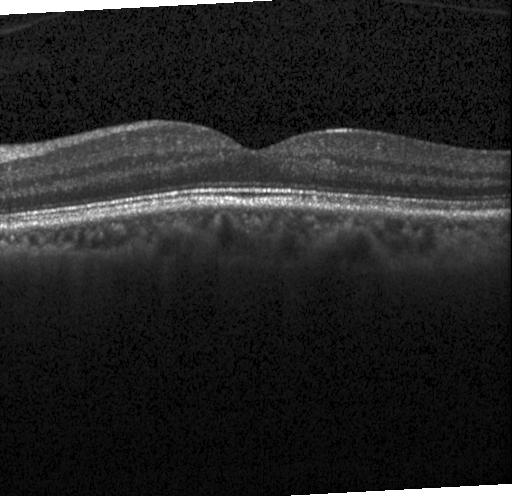

Heidelberg Spectralis OCT system · spectral-domain OCT · OCT line scan — Finding: no CNV, DME, or drusen.